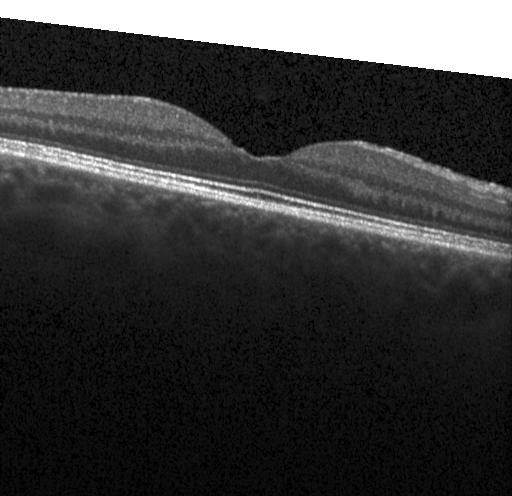
OCT finding: no evidence of choroidal neovascularization, diabetic macular edema, or drusen.